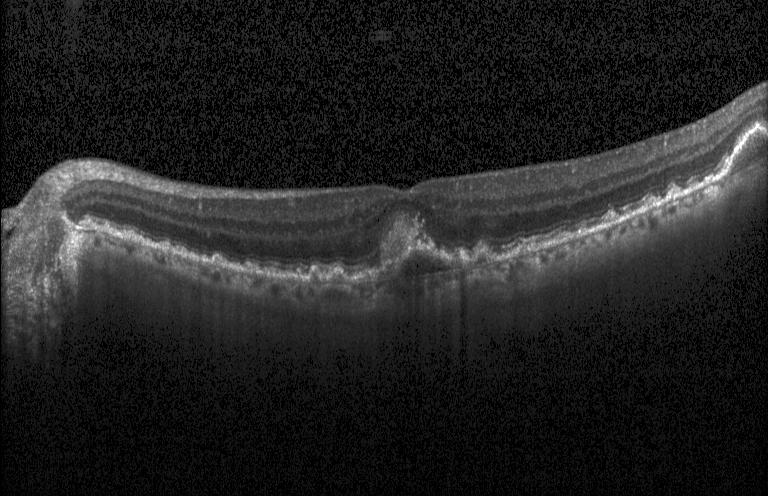
Optical coherence tomography B-scan
Assessment: choroidal neovascularization.